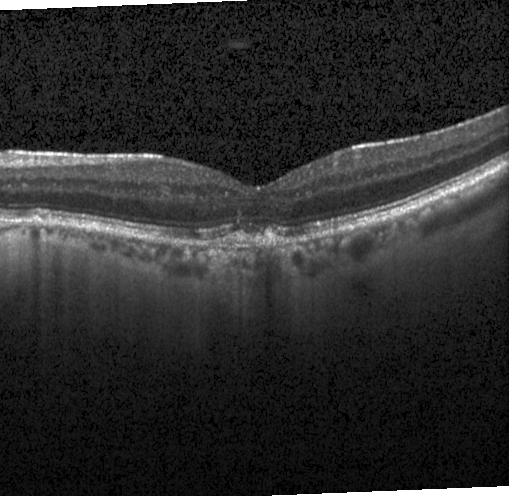
Spectral-domain optical coherence tomography, Heidelberg Spectralis OCT system, horizontal scan through the fovea, OCT B-scan — The scan shows a choroidal neovascular membrane.